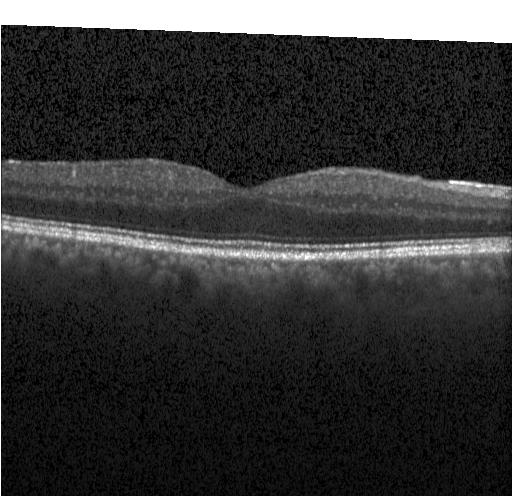 Finding: no choroidal neovascularization, no diabetic macular edema, and no drusen.